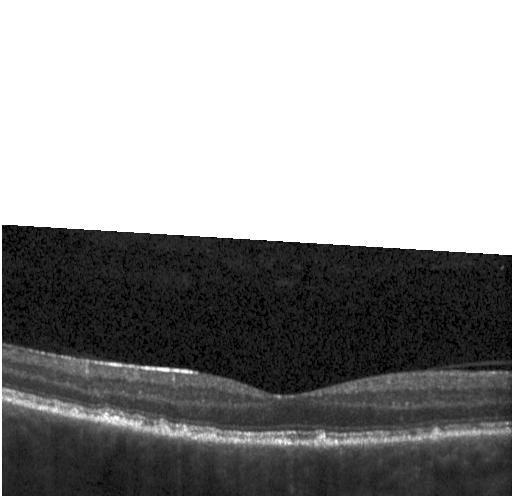

Retinal OCT cross-section showing multiple drusen.